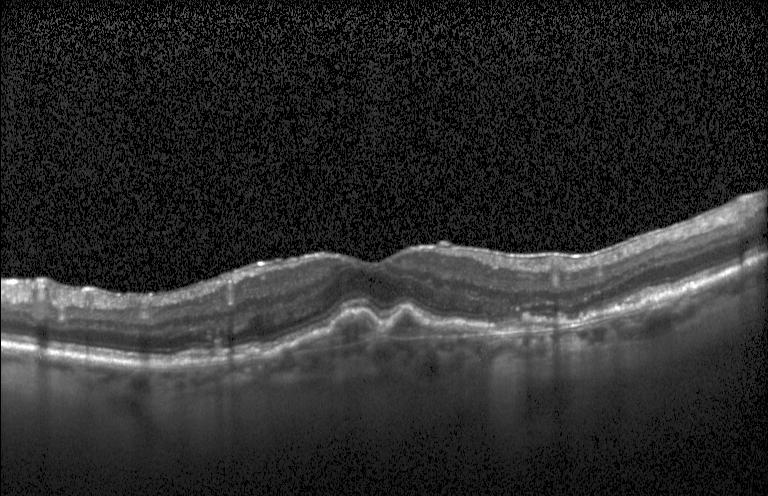

Optical coherence tomography B-scan; spectral-domain OCT; centered on the fovea — Impression: a choroidal neovascular membrane.